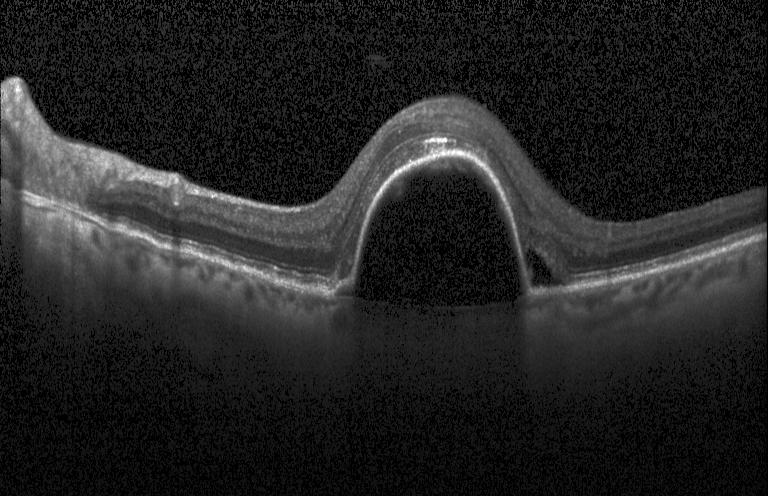

Acquired on a Heidelberg Spectralis · SD-OCT · optical coherence tomography scan · macular scan. This B-scan demonstrates CNV.